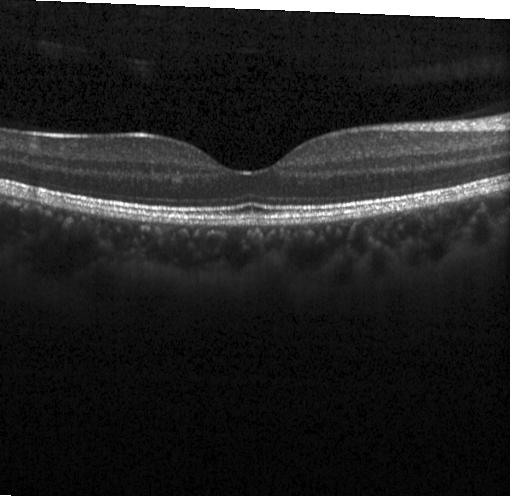

Retinal OCT cross-section — Dx: neither choroidal neovascularization, diabetic macular edema, nor drusen.